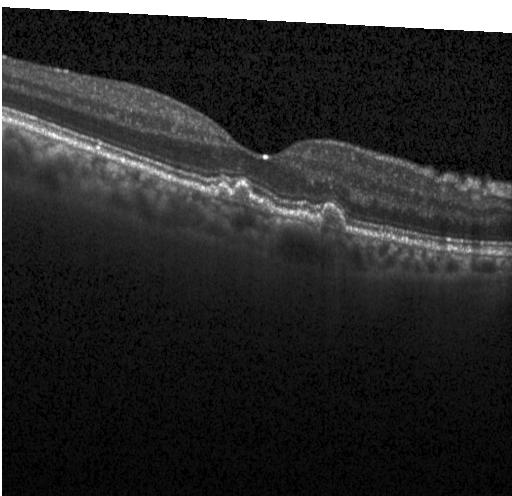 Acquired on a Heidelberg Spectralis · centered on the fovea · optical coherence tomography B-scan · SD-OCT. Impression: drusen.